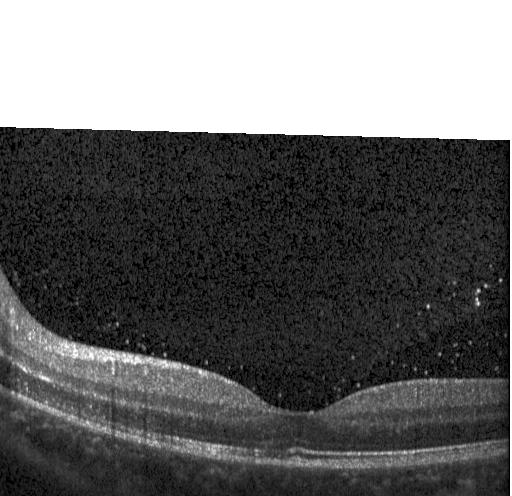
SD-OCT; through the macula; OCT line scan; Heidelberg Spectralis OCT system — Dx: no choroidal neovascularization, diabetic macular edema, or drusen.